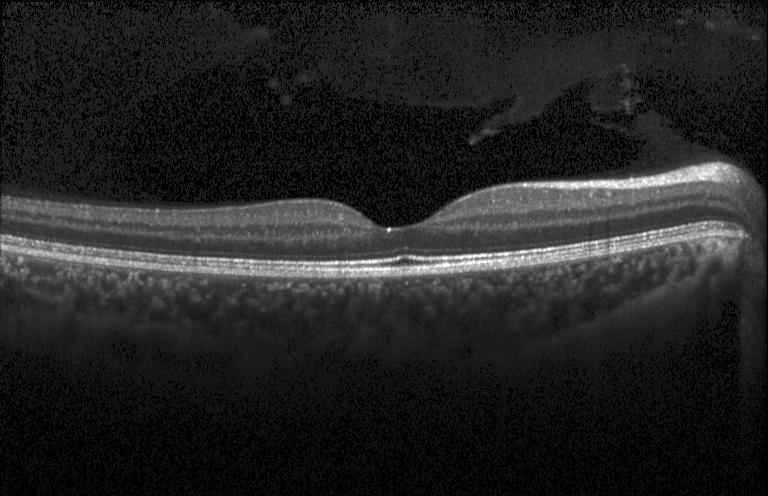
Spectral-domain OCT. Retinal OCT cross-section. Heidelberg Spectralis. The scan shows neither CNV, DME, nor drusen.